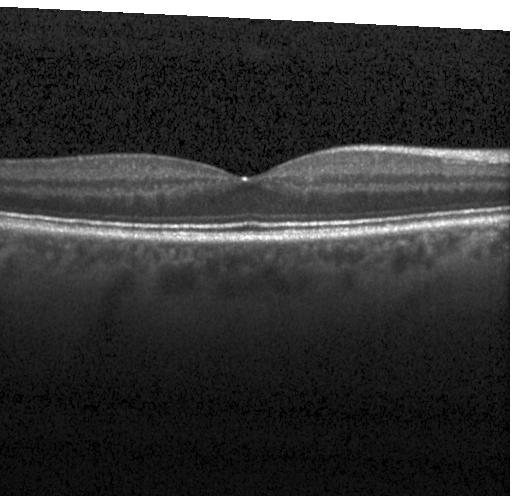 Spectral-domain OCT B-scan: no choroidal neovascularization, no diabetic macular edema, and no drusen.